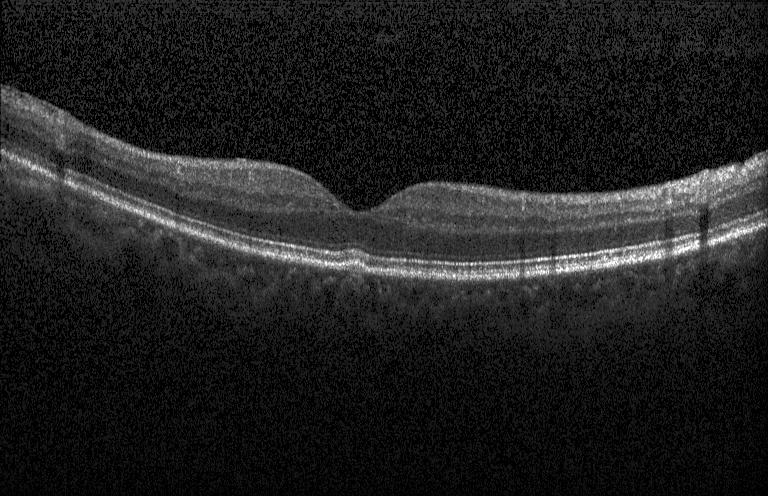

Instrument: Heidelberg Spectralis · retinal OCT B-scan · SD-OCT.
OCT finding: multiple drusen.